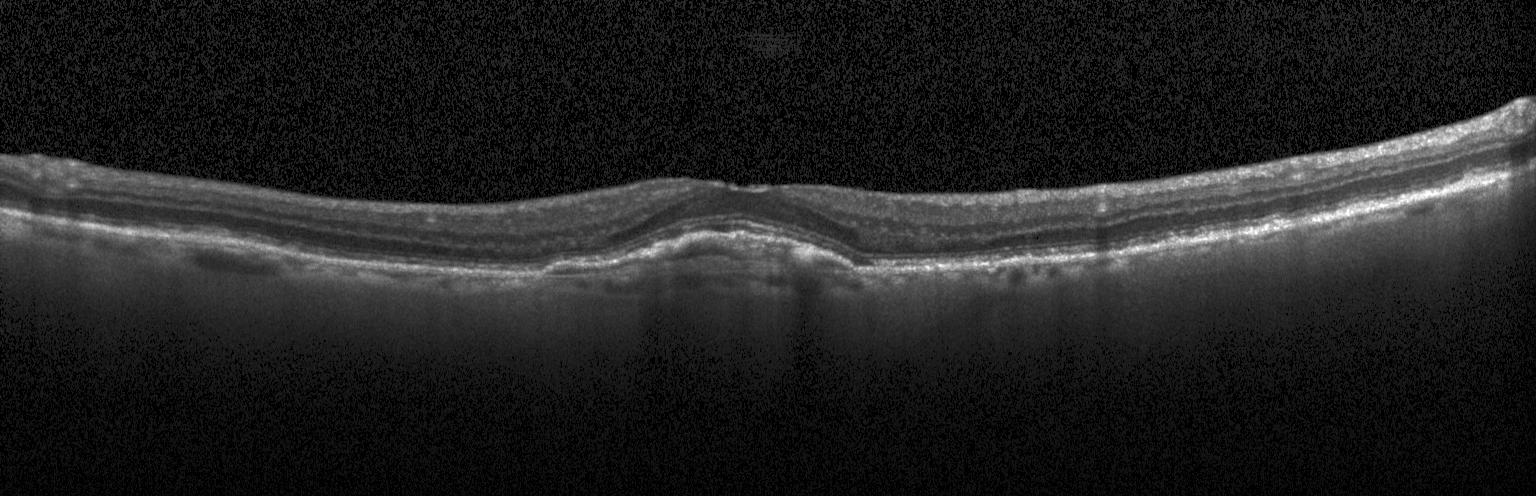
SD-OCT, optical coherence tomography B-scan, Heidelberg Spectralis OCT system, horizontal scan through the fovea. Impression: a choroidal neovascular membrane.